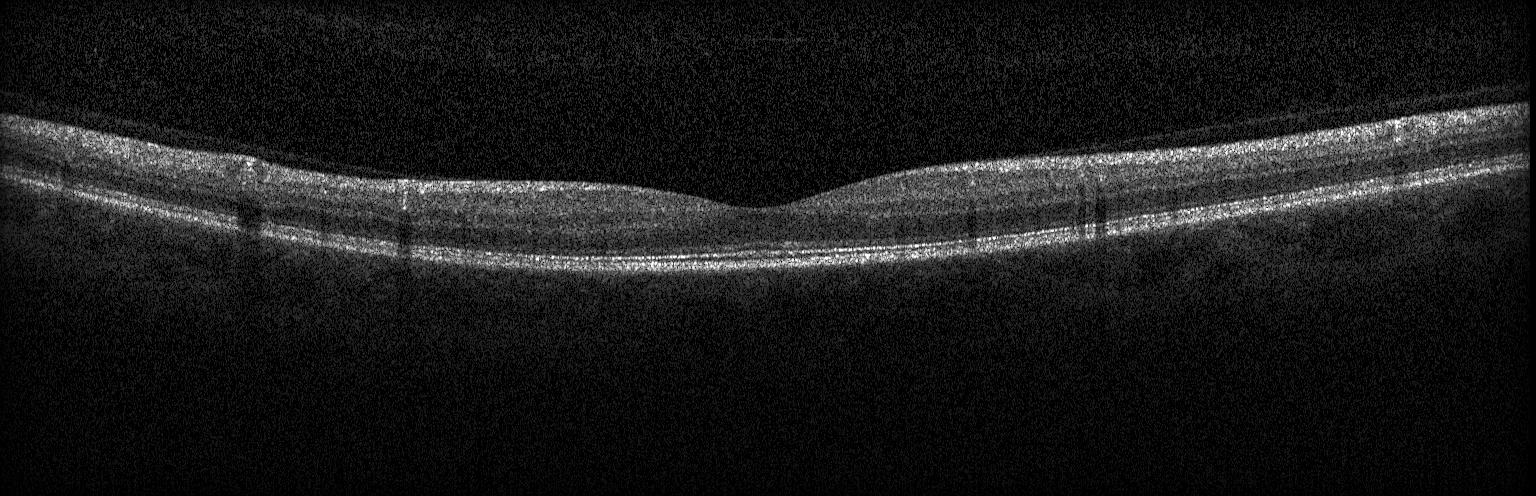 Macular OCT: no CNV, no DME, and no drusen.